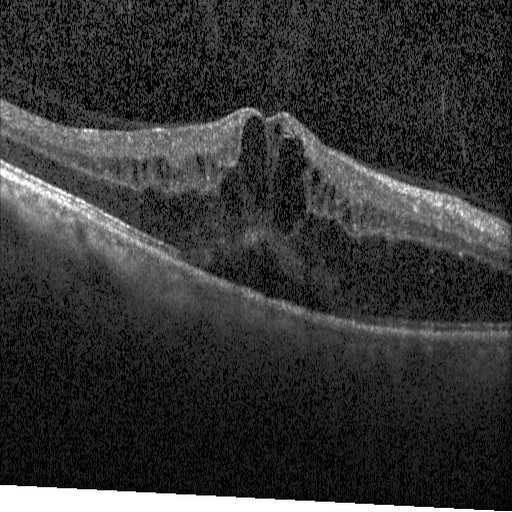 Retinal OCT cross-section. Diagnosis: DME.